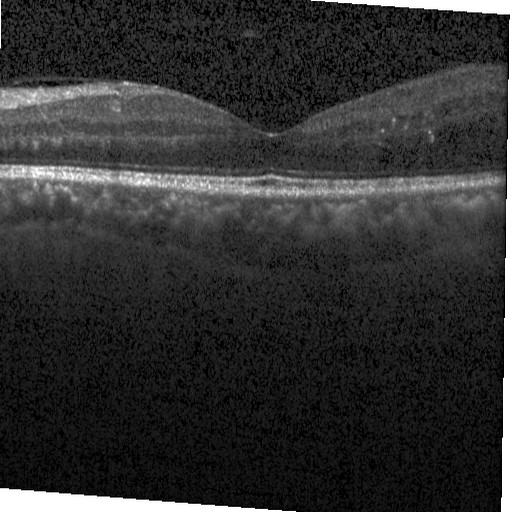 Assessment: diabetic macular edema (DME).